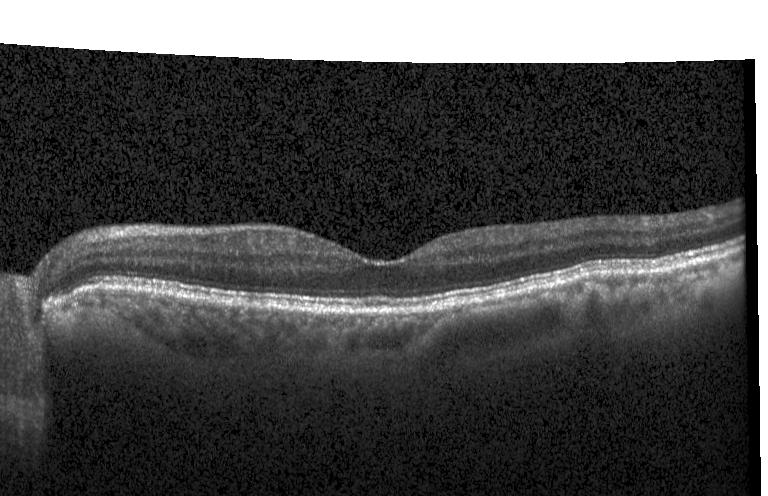
OCT scan showing no evidence of choroidal neovascularization, diabetic macular edema, or drusen.